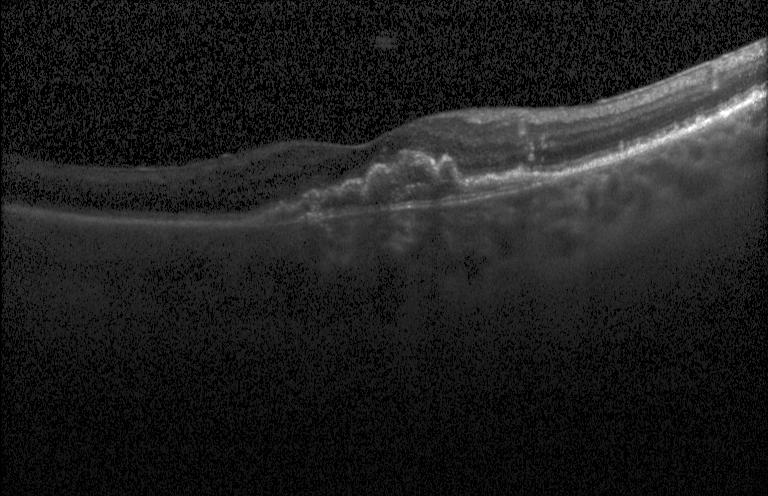
Spectral-domain OCT, Heidelberg Spectralis OCT system, optical coherence tomography B-scan
Impression: a choroidal neovascular membrane.